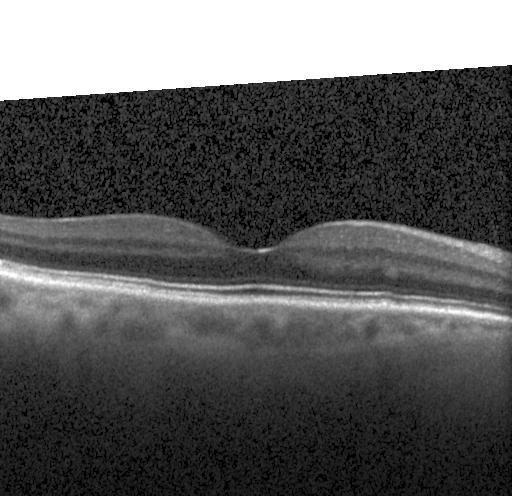
Optical coherence tomography B-scan. Spectral-domain OCT — Assessment: neither choroidal neovascularization, diabetic macular edema, nor drusen.